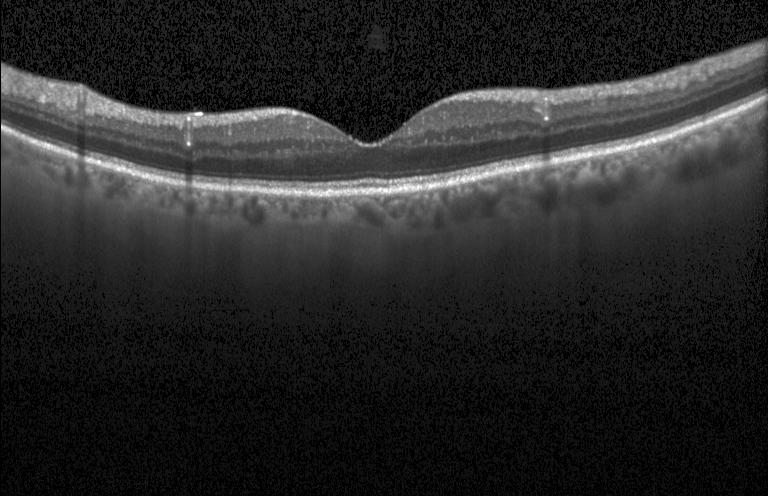 Optical coherence tomography B-scan, spectral-domain OCT. Finding: no choroidal neovascularization, no diabetic macular edema, and no drusen.